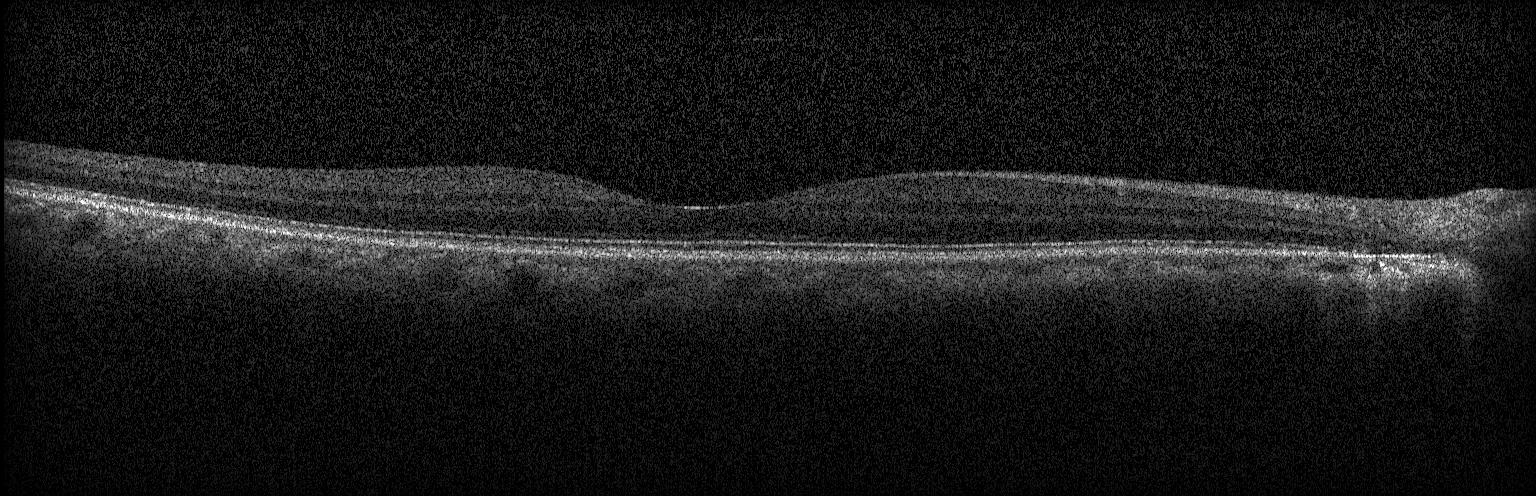 Optical coherence tomography scan; centered on the fovea; SD-OCT. Assessment: neither choroidal neovascularization, diabetic macular edema, nor drusen.